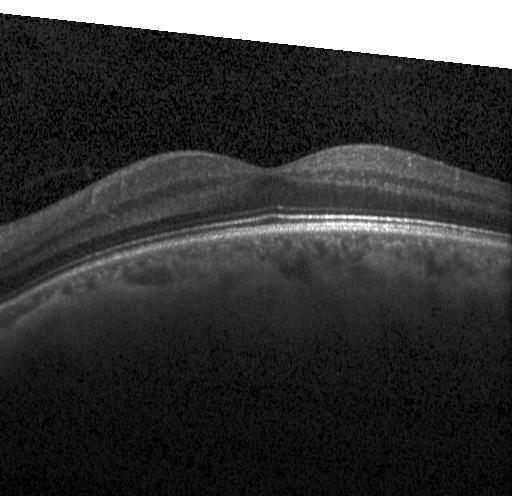

Assessment: no choroidal neovascularization, diabetic macular edema, or drusen.